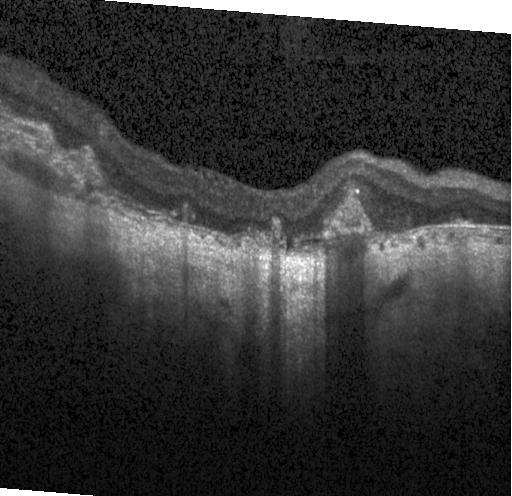 The scan shows CNV.